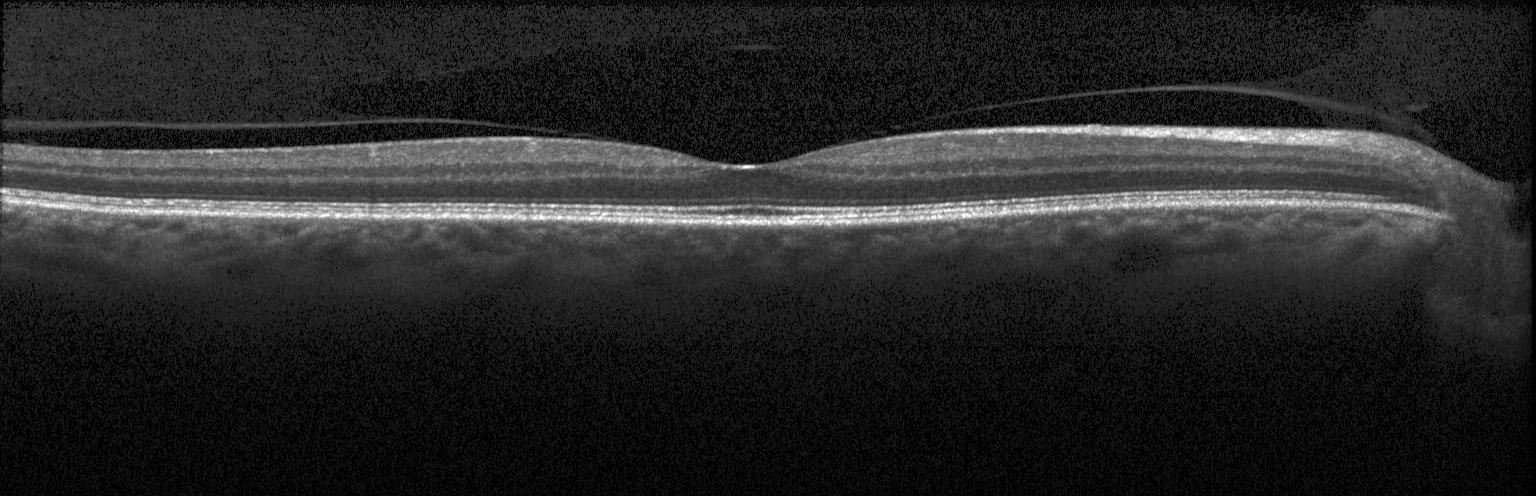 Macular OCT demonstrating no choroidal neovascularization, no diabetic macular edema, and no drusen.